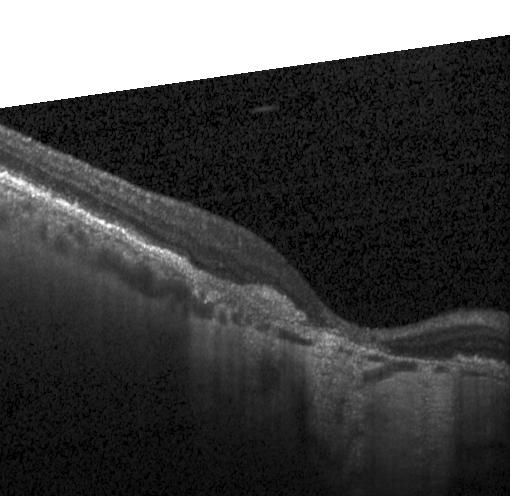

Finding: CNV.